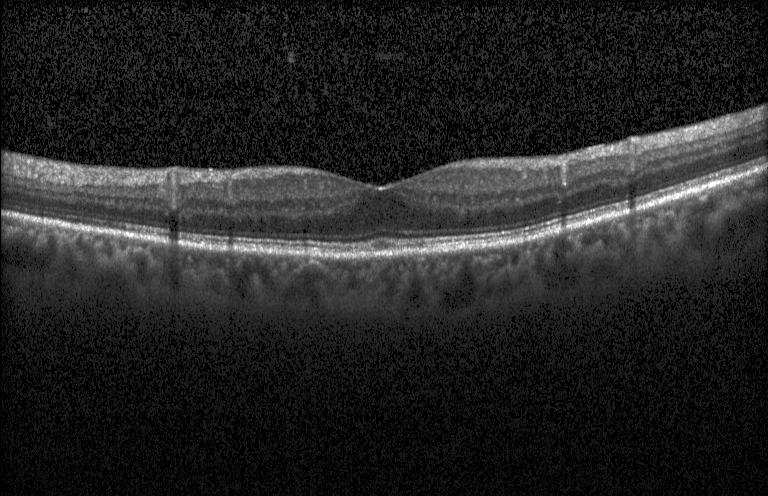
Through the macula, Heidelberg Spectralis OCT system, OCT B-scan
OCT finding: no evidence of choroidal neovascularization, diabetic macular edema, or drusen.